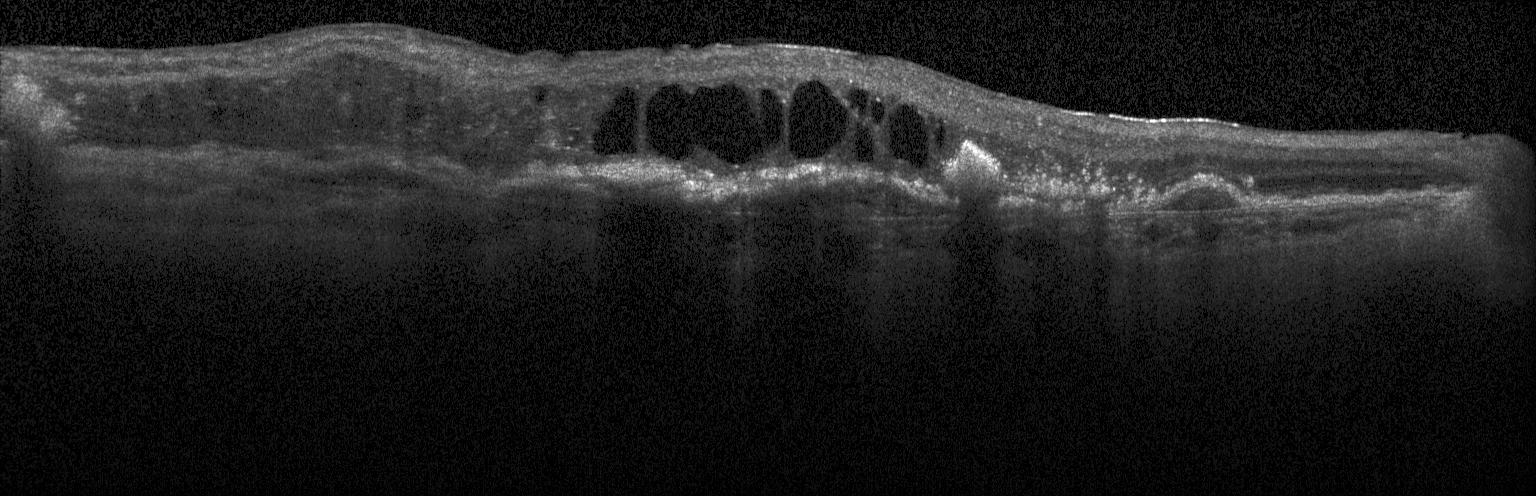
Finding: a choroidal neovascular membrane.